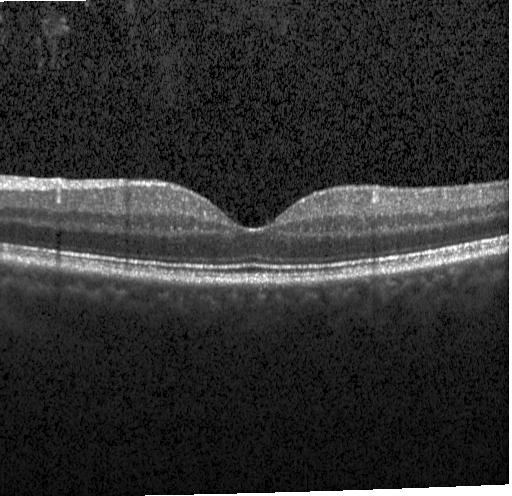 Impression: neither choroidal neovascularization, diabetic macular edema, nor drusen.